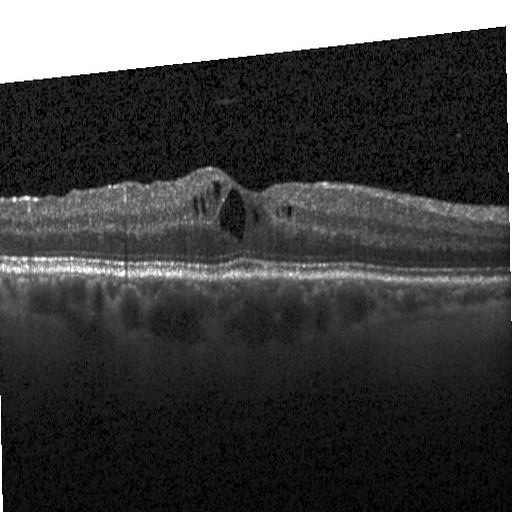
Optical coherence tomography scan — Macular OCT: diabetic macular edema (DME).